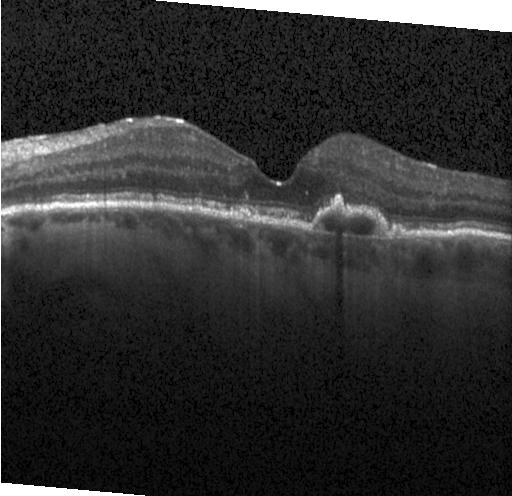

Optical coherence tomography scan.
Diagnosis: a choroidal neovascular membrane.